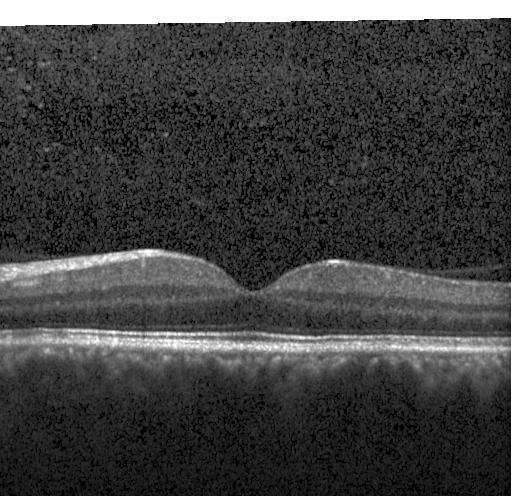 Diagnosis: no evidence of choroidal neovascularization, diabetic macular edema, or drusen.